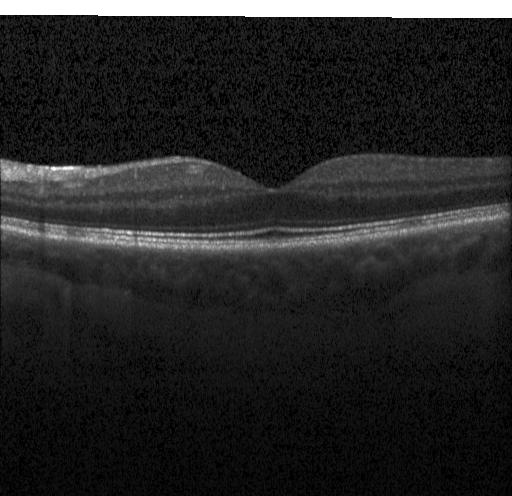 OCT line scan — Assessment: no choroidal neovascularization, no diabetic macular edema, and no drusen.